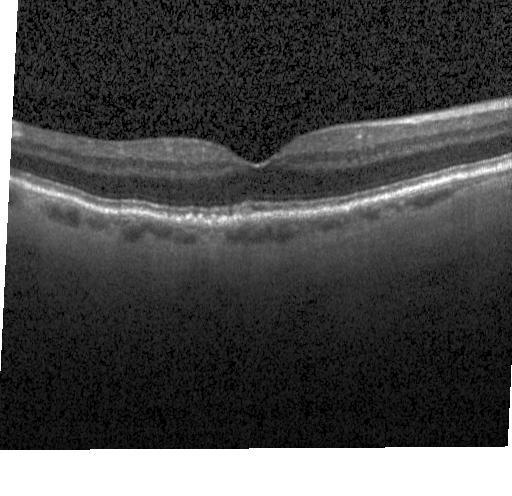 The scan shows sub-RPE drusenoid deposits.